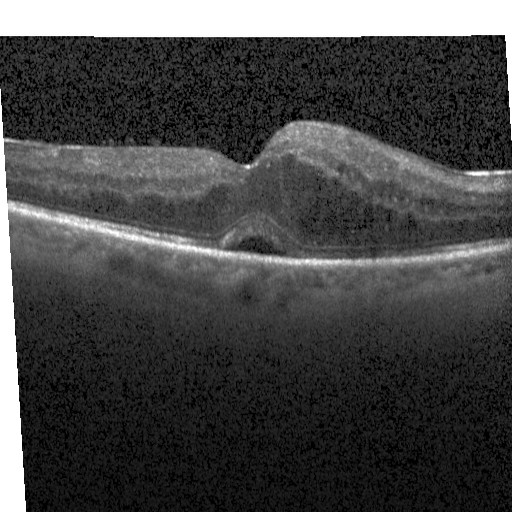
Retinal OCT B-scan · Heidelberg Spectralis · spectral-domain optical coherence tomography · centered on the fovea
Finding: diabetic macular edema (DME).